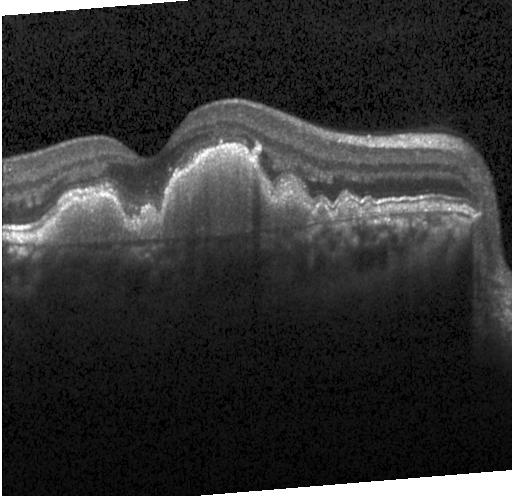 Spectral-domain OCT. Retinal OCT cross-section. Horizontal scan through the fovea
Macular OCT: drusen.